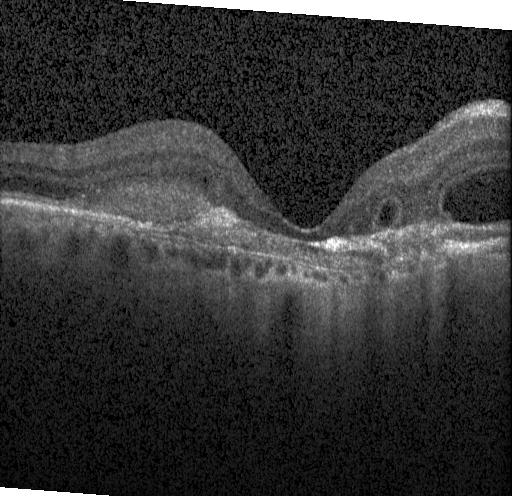

Spectral-domain optical coherence tomography; centered on the fovea; retinal OCT cross-section
Diagnosis: choroidal neovascularization (CNV).